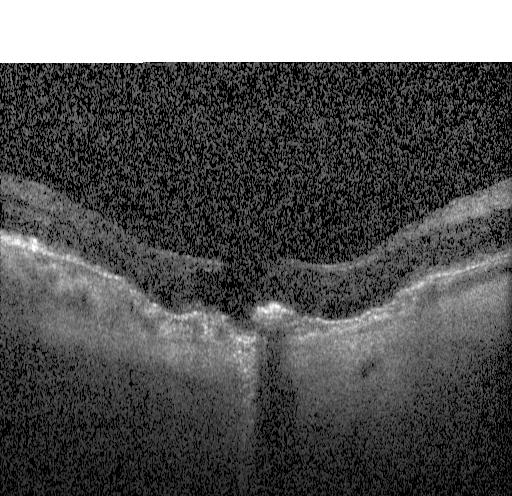

OCT line scan
Finding: CNV.